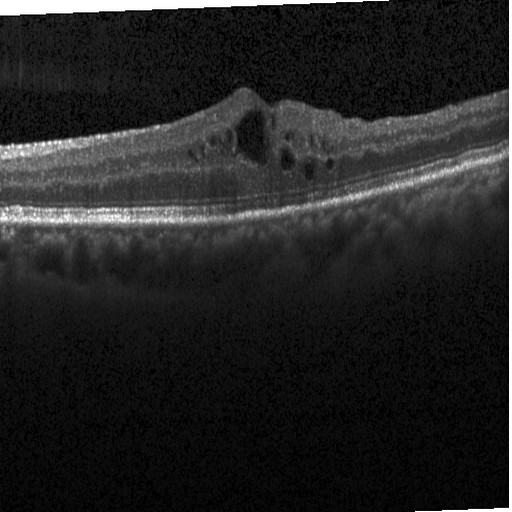

Retinal OCT cross-section showing DME.